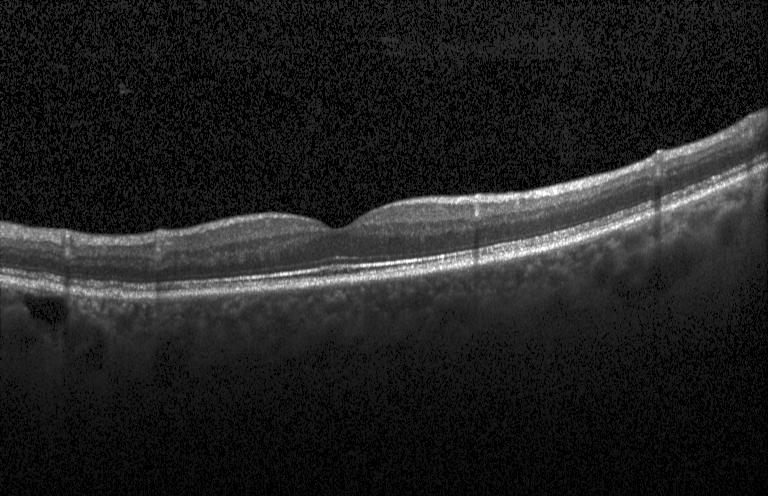 Retinal OCT cross-section. Fovea-centered. Acquired on a Heidelberg Spectralis. SD-OCT — Finding: no CNV, DME, or drusen.